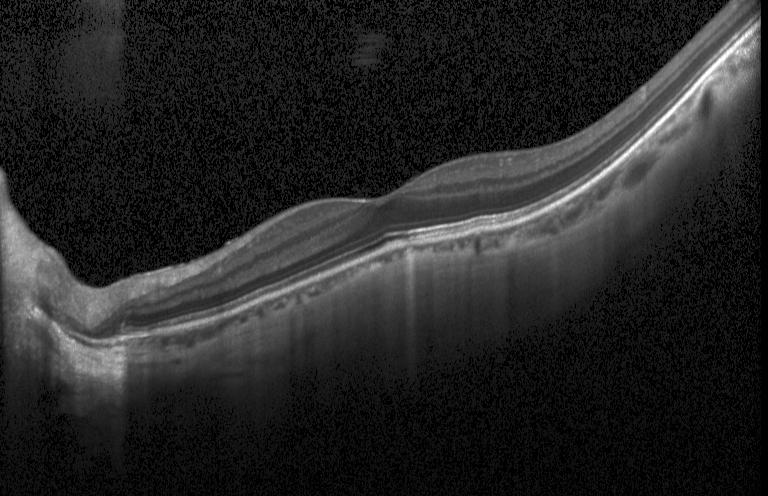
Horizontal scan through the fovea, retinal OCT cross-section. Diagnosis: no evidence of choroidal neovascularization, diabetic macular edema, or drusen.